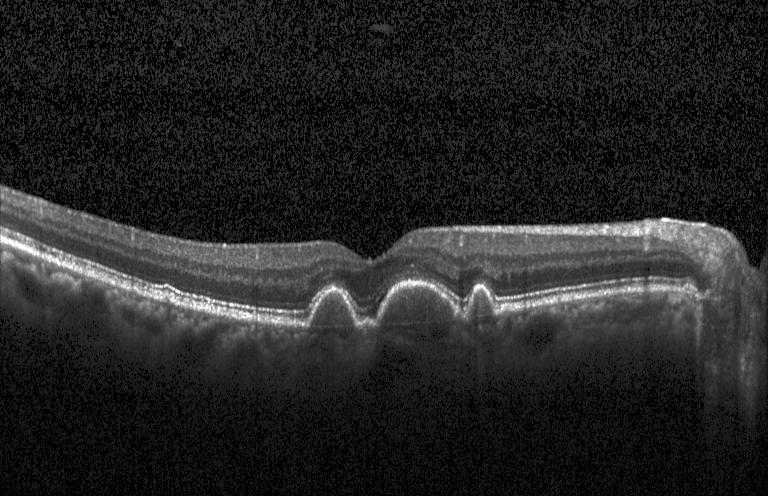 Heidelberg Spectralis. Centered on the fovea. OCT line scan
Diagnosis: drusen.